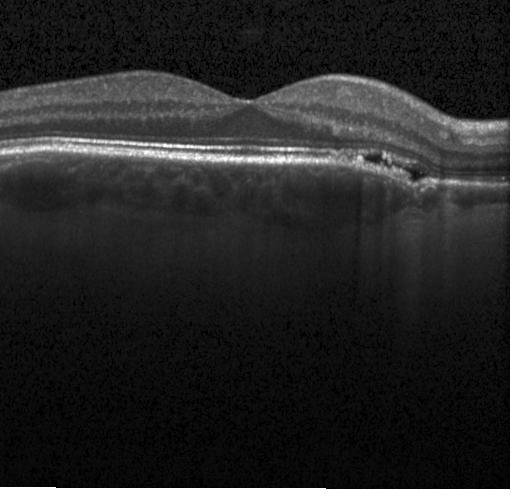
OCT B-scan showing choroidal neovascularization.